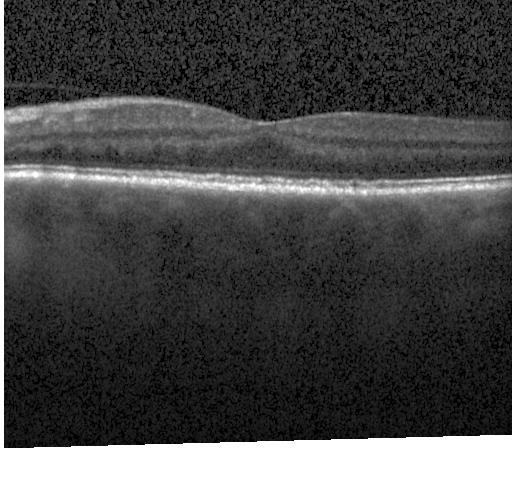 OCT B-scan
Dx: neither CNV, DME, nor drusen.